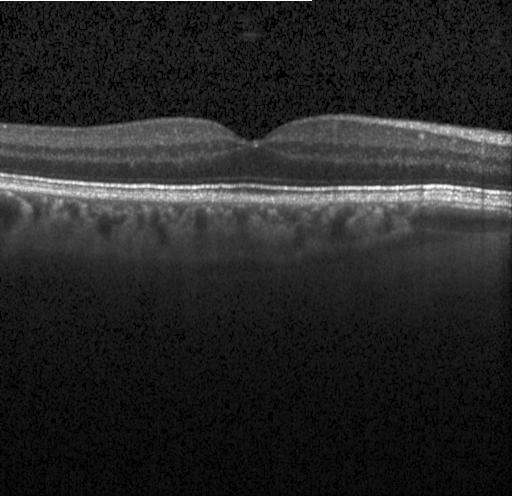
No choroidal neovascularization, no diabetic macular edema, and no drusen.